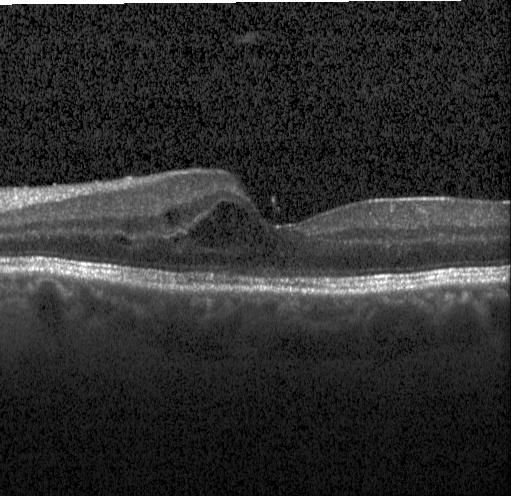
Optical coherence tomography scan; acquired on a Heidelberg Spectralis; through the macula; spectral-domain OCT. Dx: diabetic macular edema (DME).